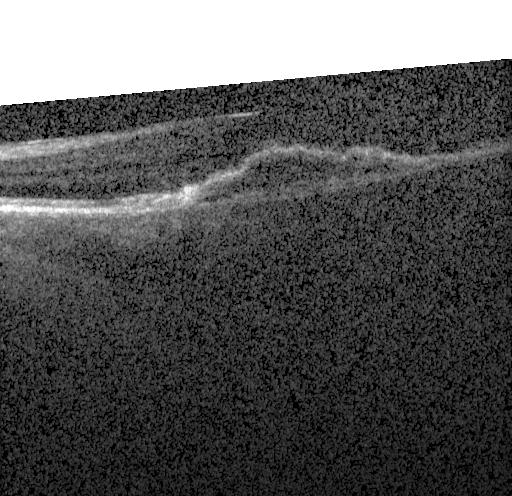
Diagnosis: a choroidal neovascular membrane.